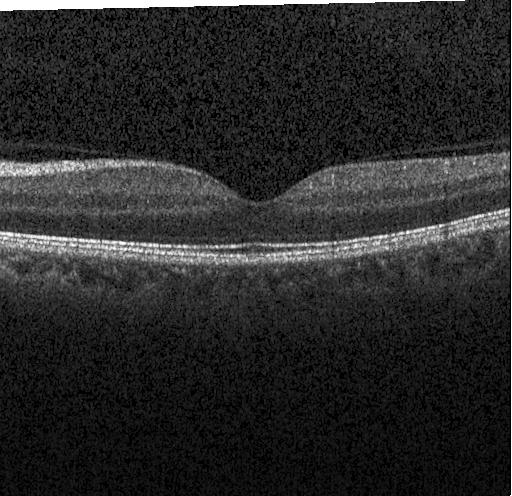 Spectral-domain optical coherence tomography; optical coherence tomography B-scan. Assessment: no CNV, no DME, and no drusen.